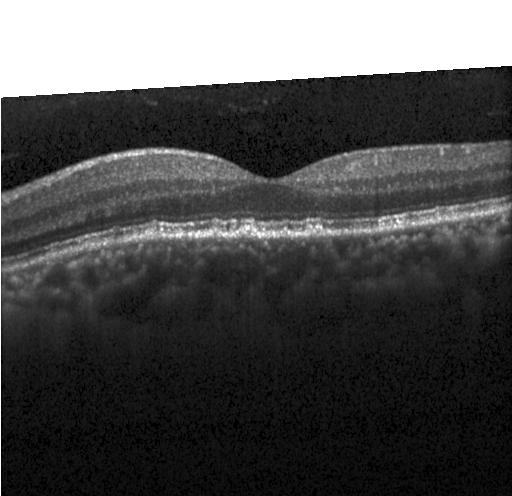

Spectral-domain OCT B-scan: drusen.